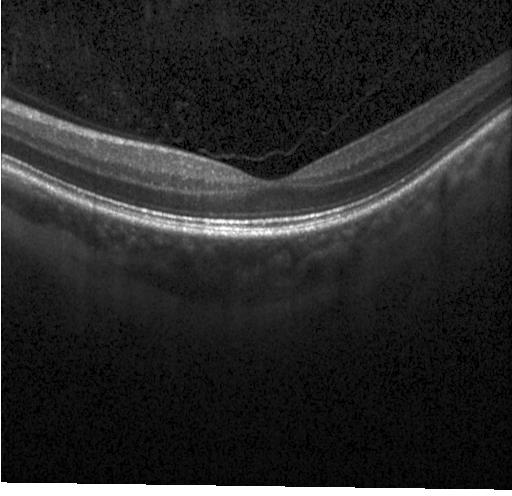 Impression: neither CNV, DME, nor drusen.